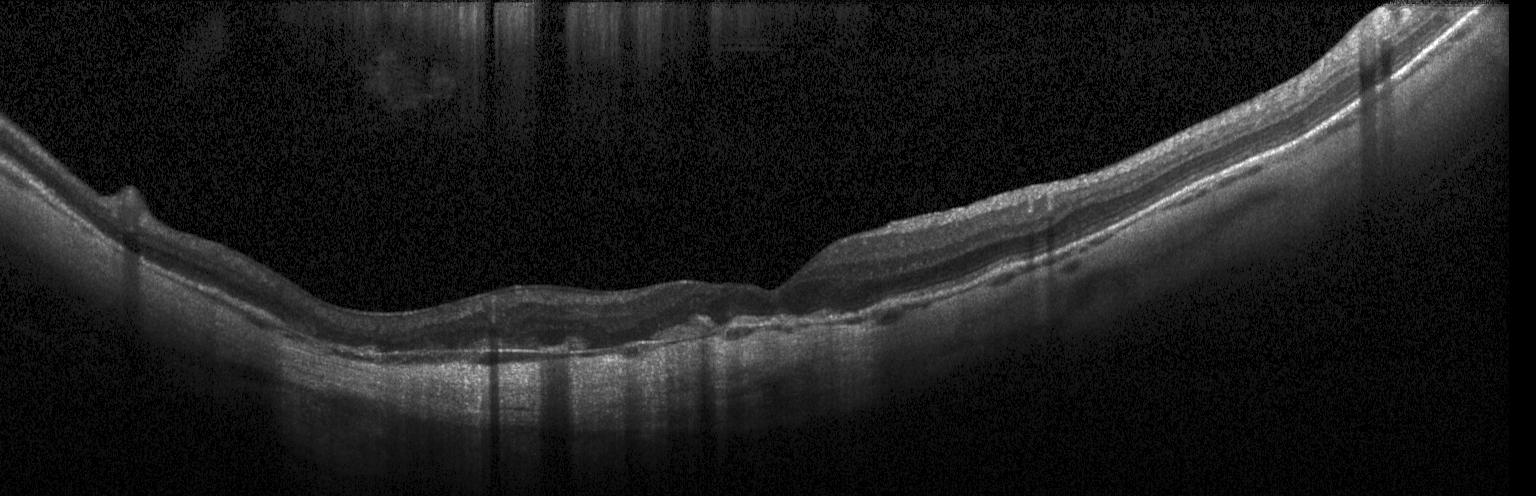

Optical coherence tomography B-scan; spectral-domain OCT.
This B-scan demonstrates a choroidal neovascular membrane.